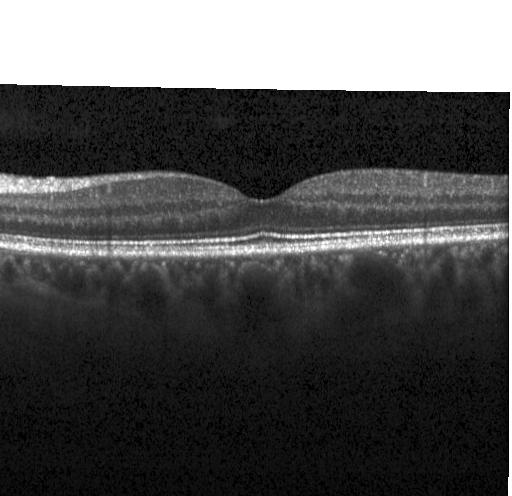 Assessment: neither CNV, DME, nor drusen.